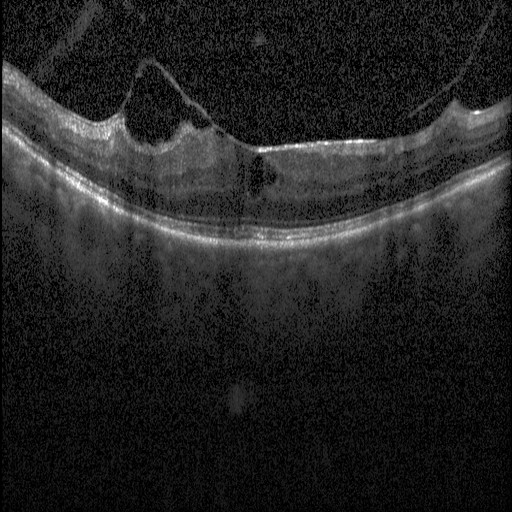

Retinal OCT cross-section
The scan shows DME.